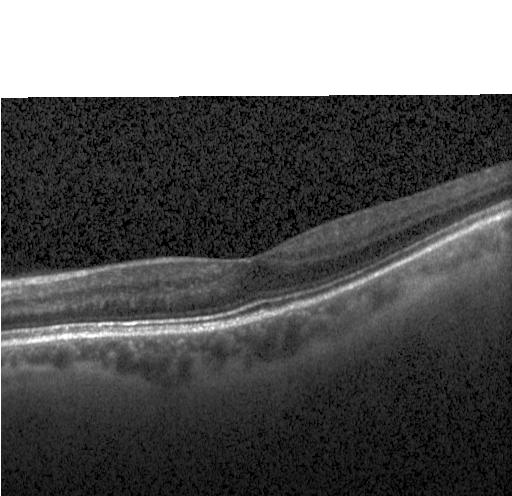 Optical coherence tomography B-scan.
Finding: no choroidal neovascularization, diabetic macular edema, or drusen.